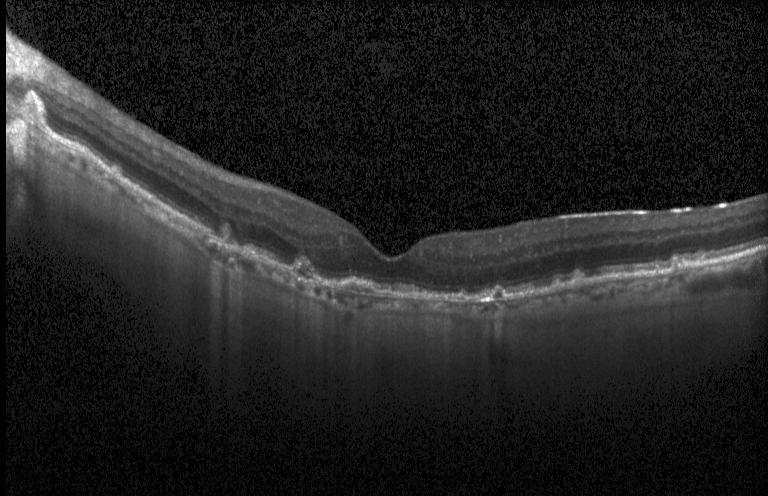
Retinal OCT B-scan.
This B-scan demonstrates CNV.